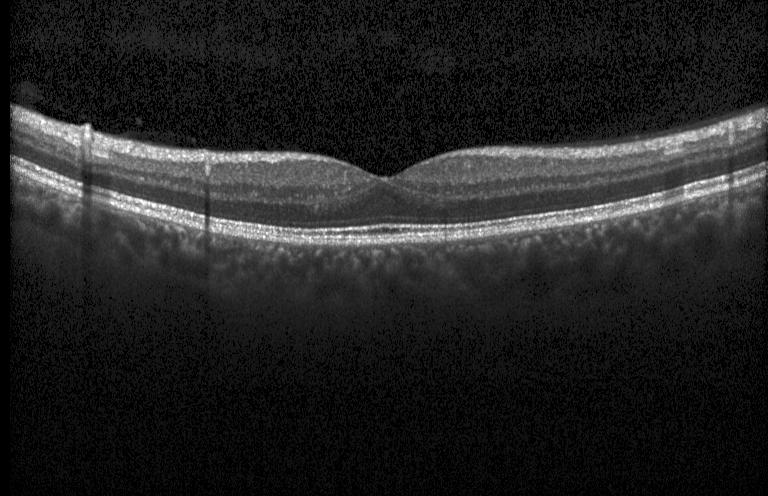 OCT line scan; centered on the fovea. Impression: no choroidal neovascularization, no diabetic macular edema, and no drusen.